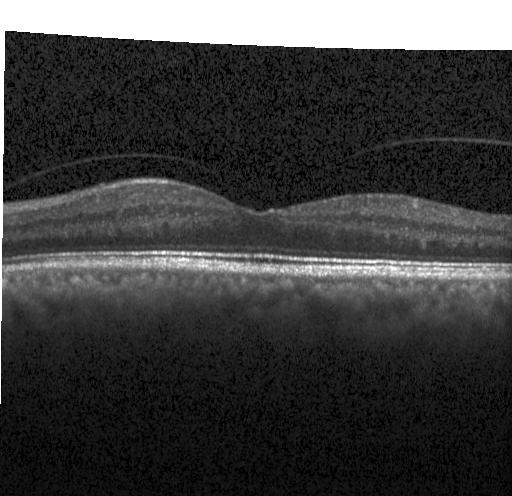

SD-OCT · instrument: Heidelberg Spectralis · optical coherence tomography B-scan · centered on the fovea. Diagnosis: neither choroidal neovascularization, diabetic macular edema, nor drusen.